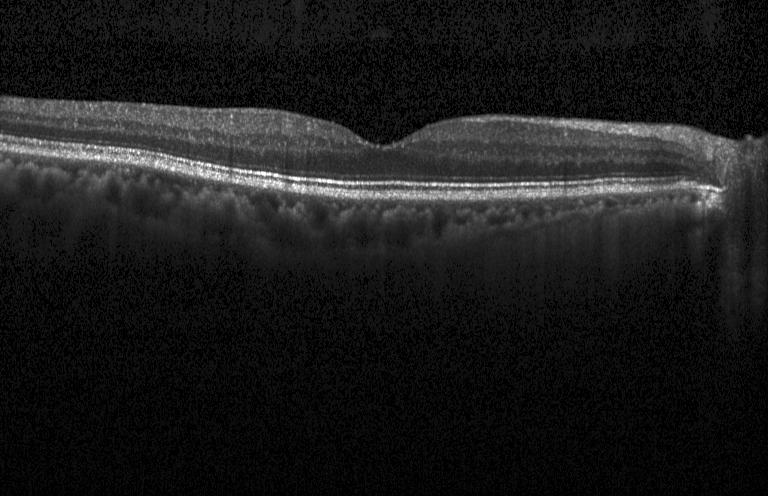 OCT finding: no evidence of CNV, DME, or drusen.